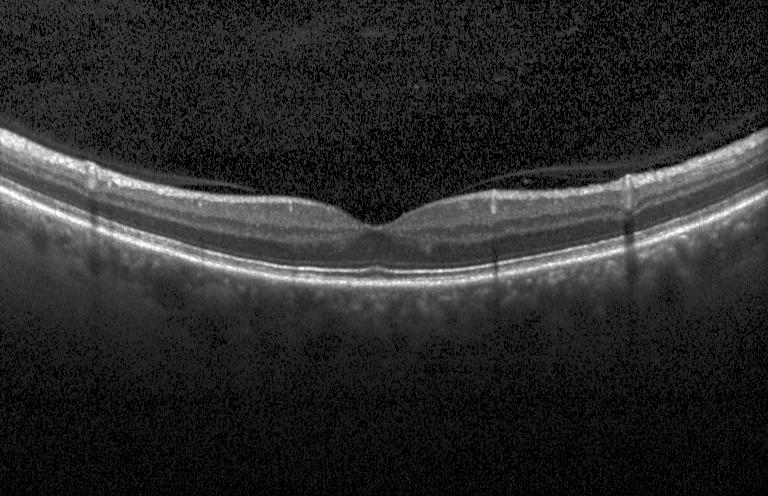

Optical coherence tomography B-scan; horizontal scan through the fovea — Impression: no CNV, DME, or drusen.